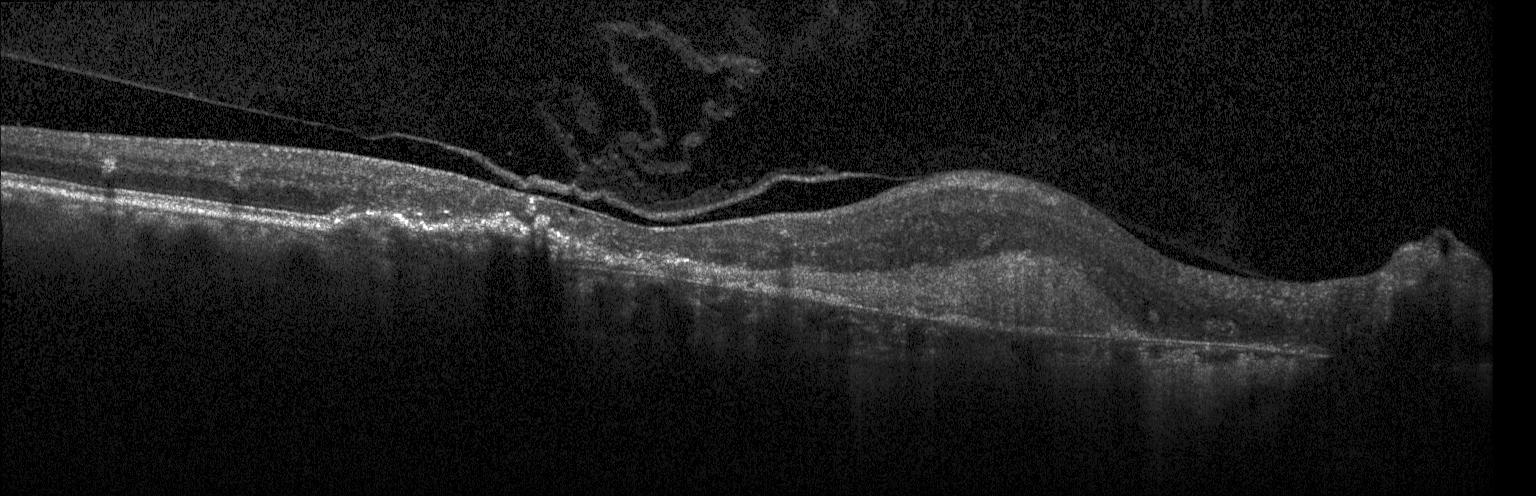

OCT B-scan · macular scan · spectral-domain optical coherence tomography — Diagnosis: choroidal neovascularization.